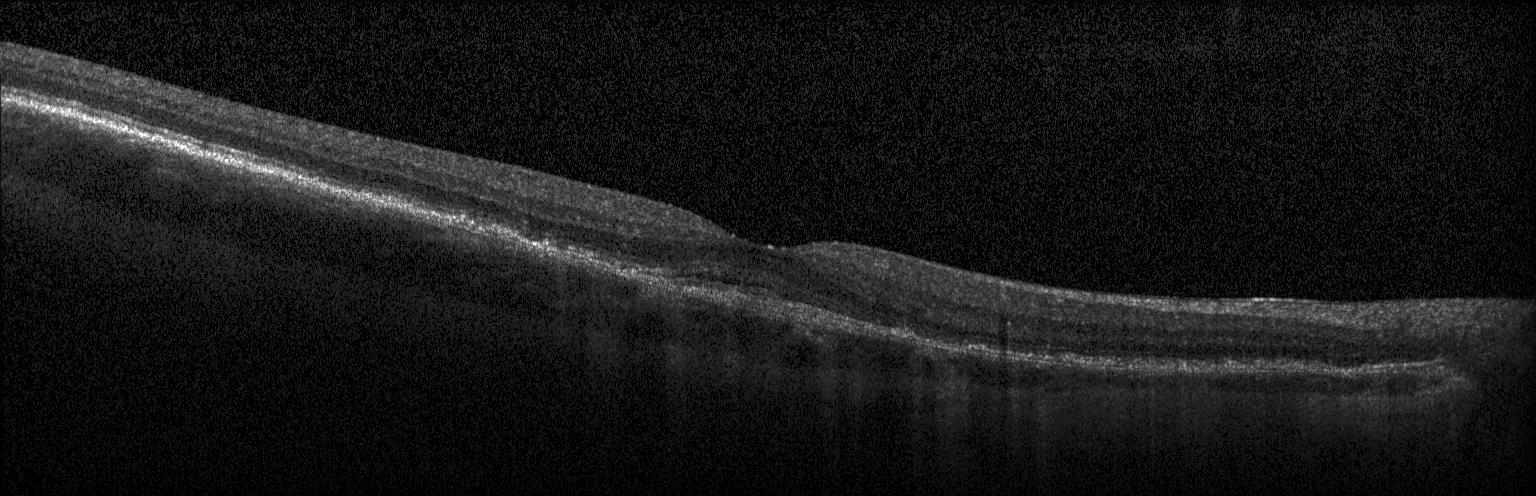

Heidelberg Spectralis OCT system · spectral-domain OCT · OCT B-scan · through the macula
The scan shows a choroidal neovascular membrane.